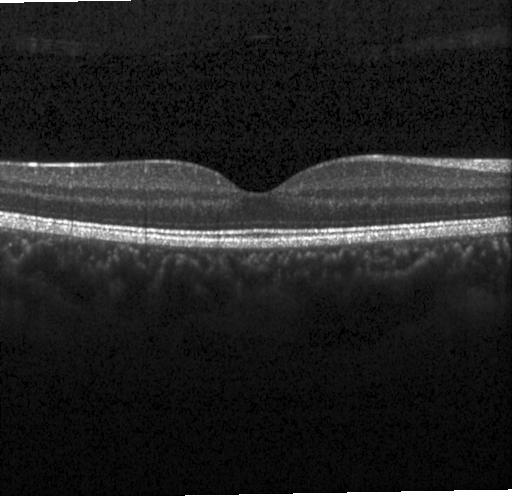 OCT scan showing no evidence of choroidal neovascularization, diabetic macular edema, or drusen.